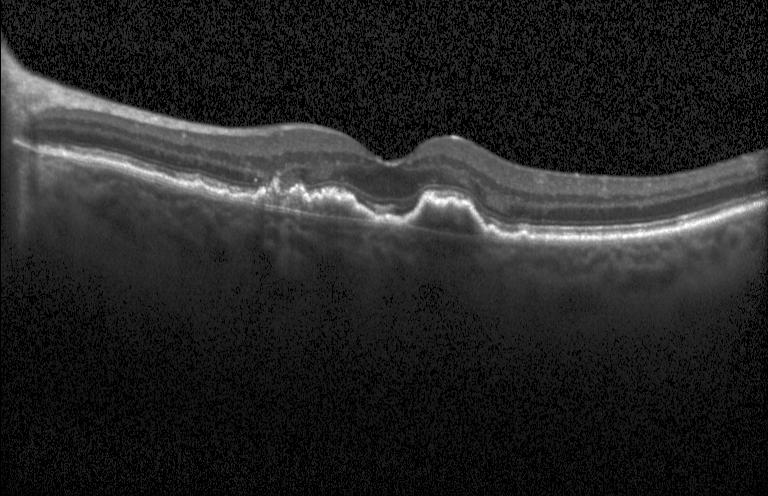

Acquired on a Heidelberg Spectralis, retinal OCT cross-section. OCT finding: a choroidal neovascular membrane.